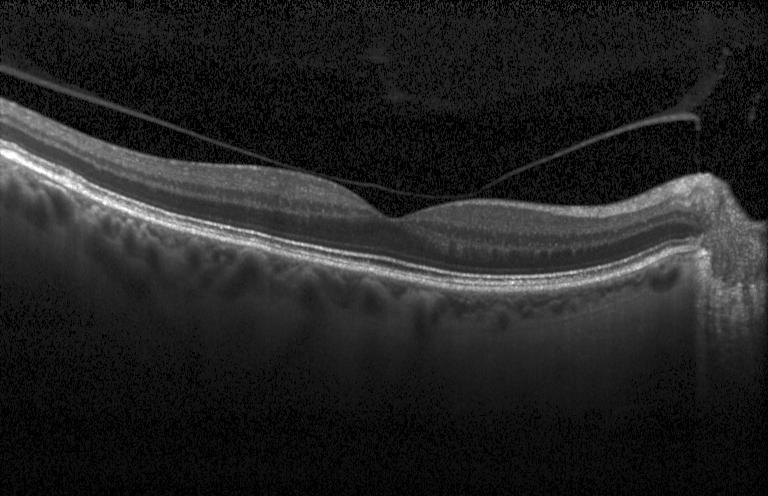 Retinal OCT cross-section showing neither choroidal neovascularization, diabetic macular edema, nor drusen.